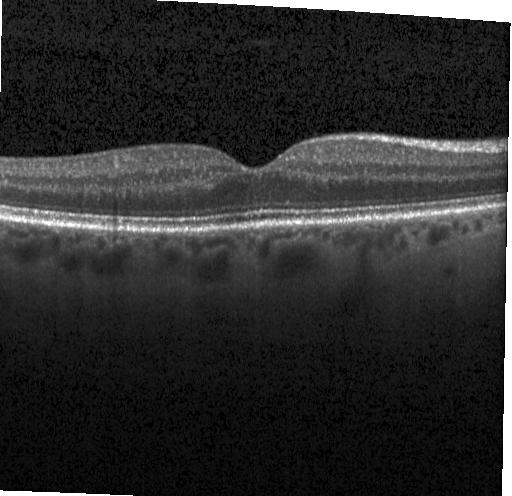 OCT B-scan. Spectral-domain optical coherence tomography. Acquired on a Heidelberg Spectralis.
The scan shows no evidence of choroidal neovascularization, diabetic macular edema, or drusen.